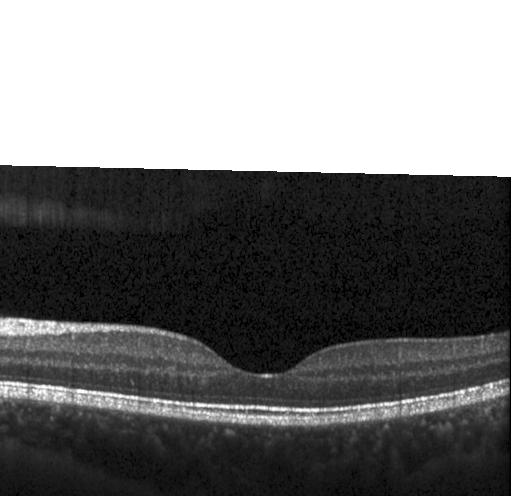
Impression: no choroidal neovascularization, diabetic macular edema, or drusen.